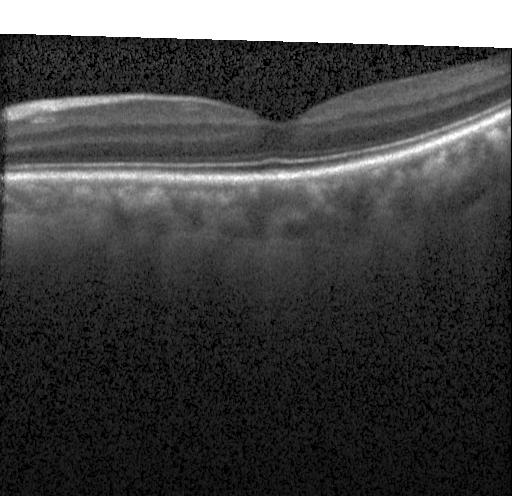 Optical coherence tomography B-scan
OCT finding: neither CNV, DME, nor drusen.